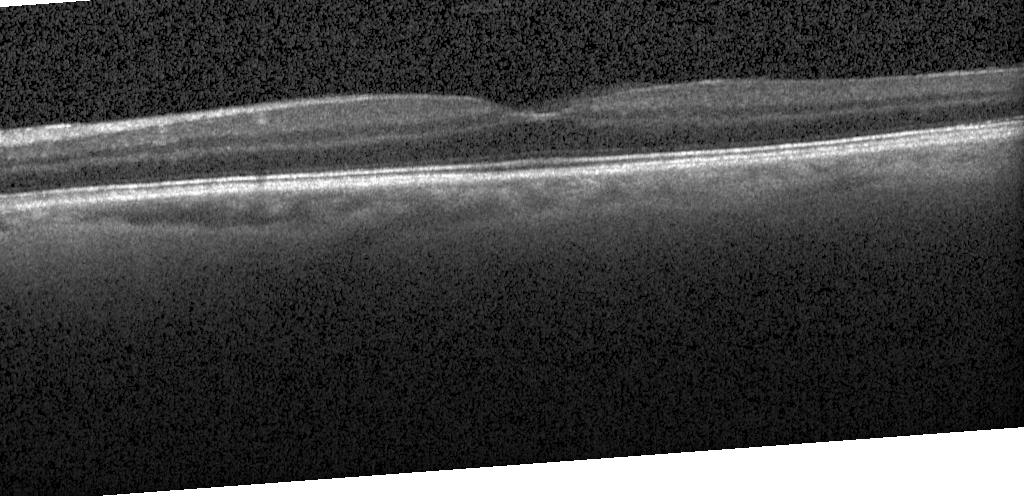

OCT B-scan; acquired on a Heidelberg Spectralis — The scan shows no CNV, DME, or drusen.